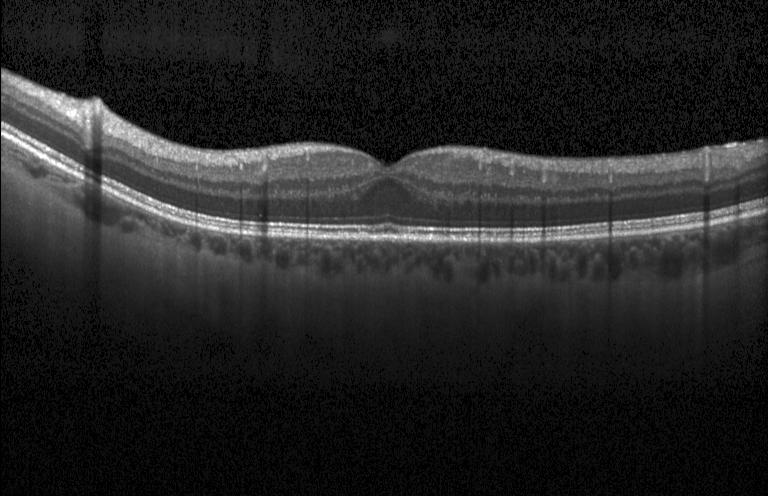

OCT scan showing no choroidal neovascularization, diabetic macular edema, or drusen.